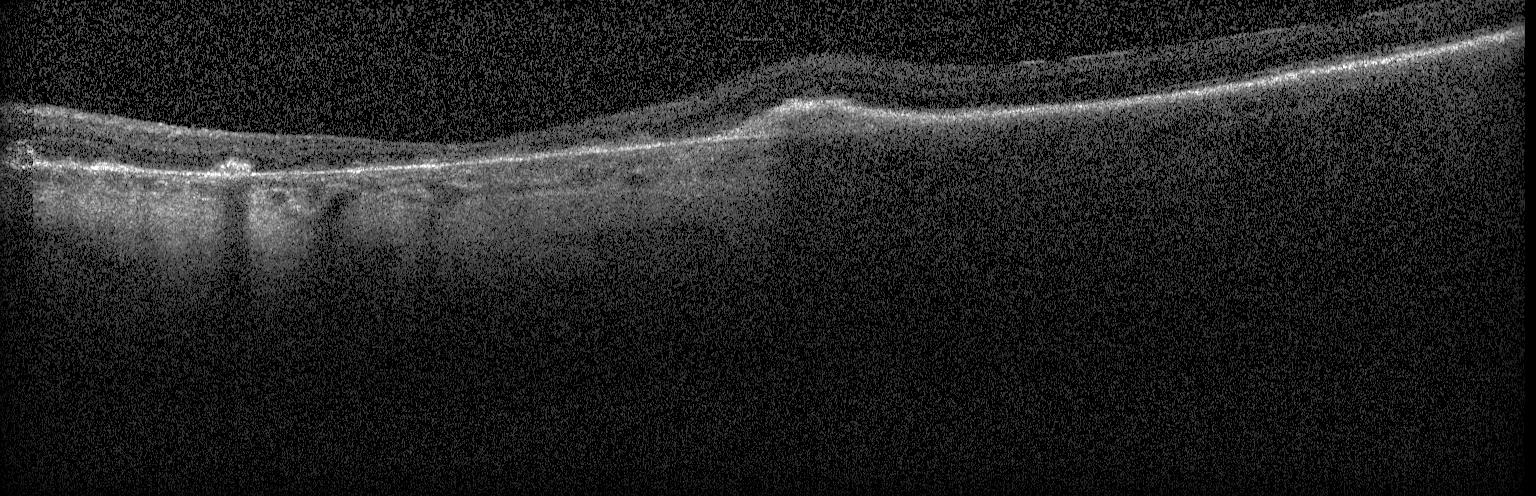
Spectral-domain optical coherence tomography. Fovea-centered. Acquired on a Heidelberg Spectralis. Retinal OCT B-scan
This B-scan demonstrates choroidal neovascularization (CNV).